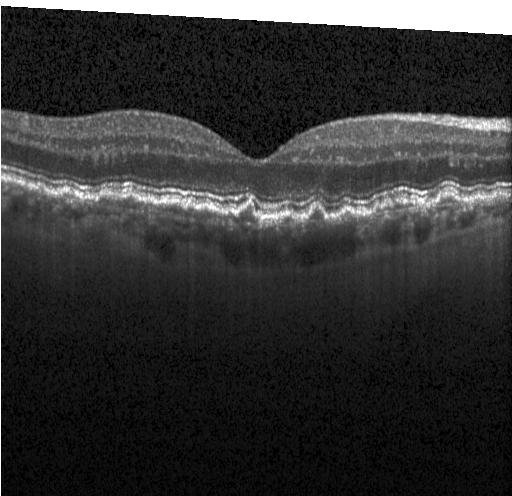
Impression: multiple drusen.